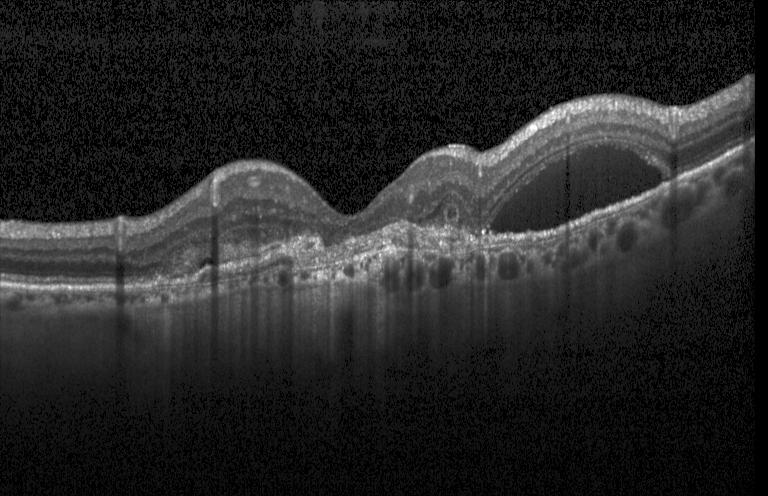 Impression: a choroidal neovascular membrane.